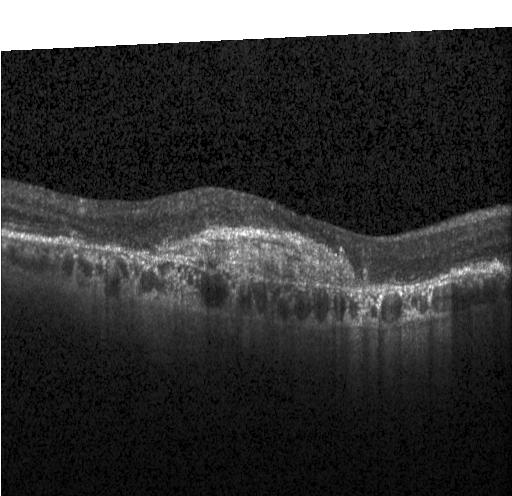

OCT scan showing a choroidal neovascular membrane.